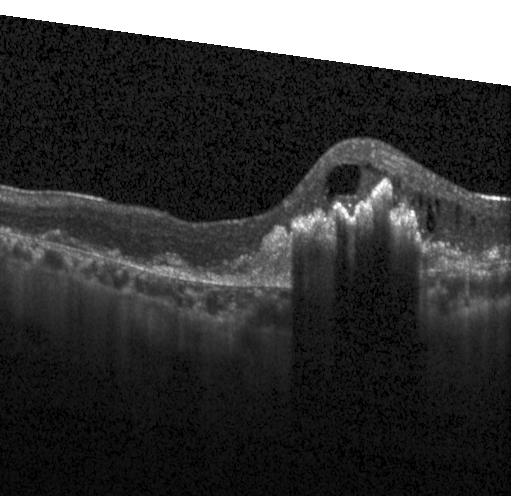 OCT B-scan showing a choroidal neovascular membrane.